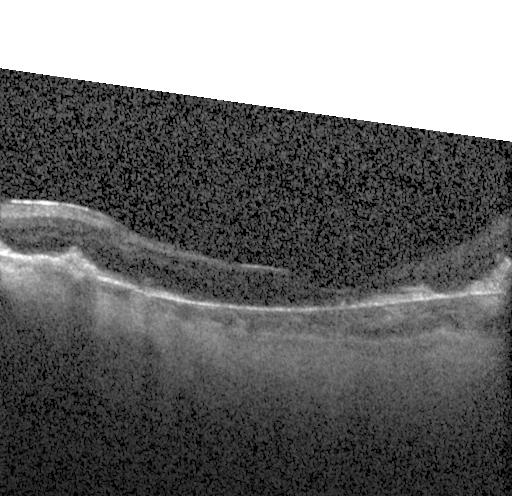

SD-OCT; Heidelberg Spectralis OCT system; retinal OCT cross-section
The scan shows CNV.